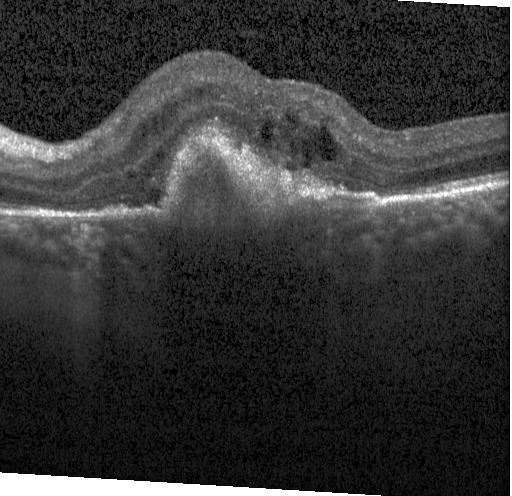

Retinal OCT cross-section, horizontal scan through the fovea, acquired on a Heidelberg Spectralis.
This B-scan demonstrates a choroidal neovascular membrane.